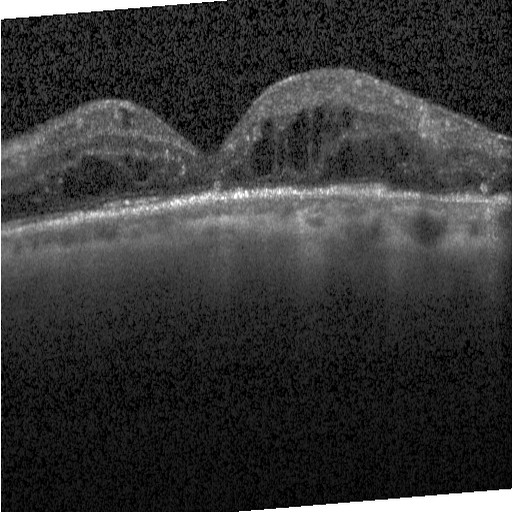
Macular scan. Optical coherence tomography scan. Spectral-domain OCT. Heidelberg Spectralis OCT system — Impression: diabetic macular edema.